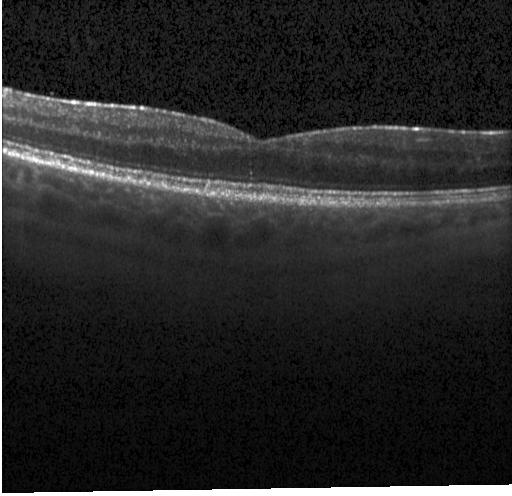 Retinal OCT B-scan
The scan shows no choroidal neovascularization, diabetic macular edema, or drusen.